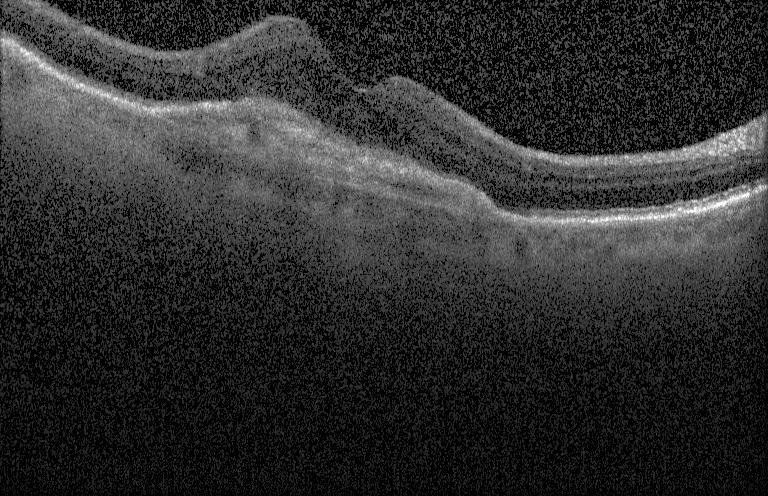

Dx: CNV.